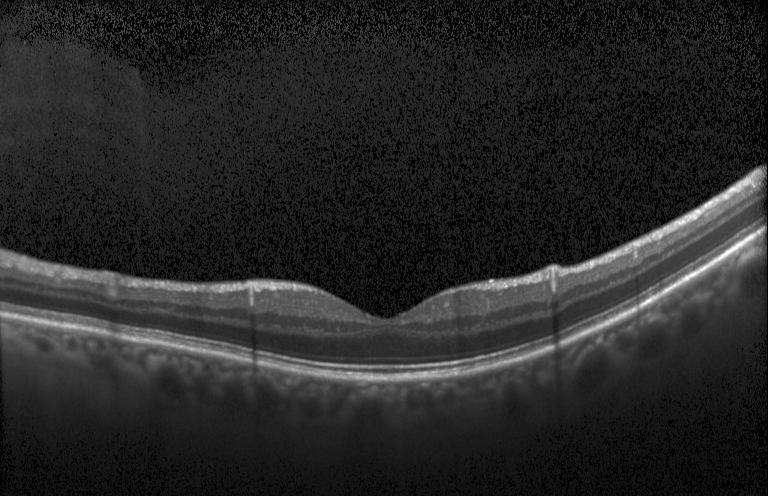

Optical coherence tomography B-scan — Diagnosis: neither CNV, DME, nor drusen.